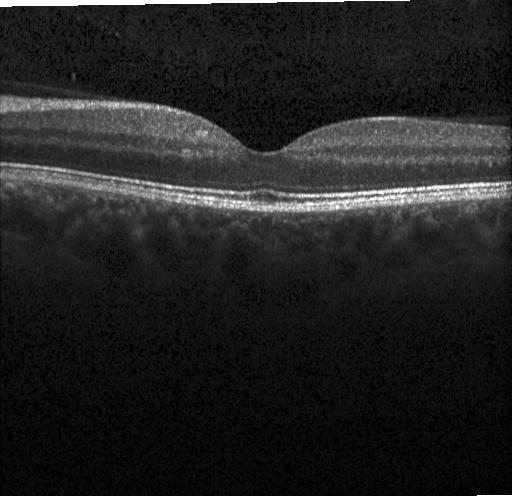 OCT line scan; centered on the fovea; Heidelberg Spectralis OCT system
Impression: neither choroidal neovascularization, diabetic macular edema, nor drusen.